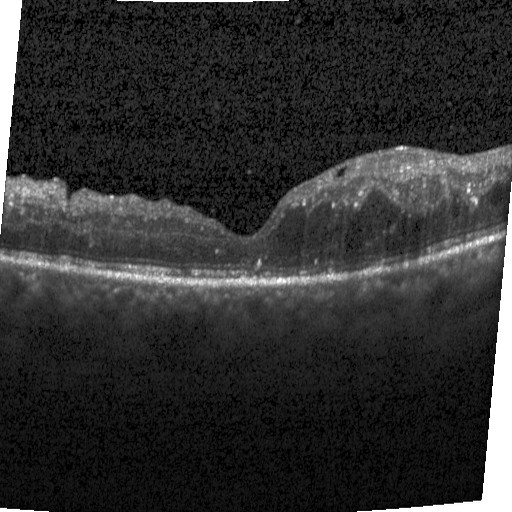

Spectral-domain OCT. Heidelberg Spectralis. Retinal OCT cross-section
Macular OCT: DME.